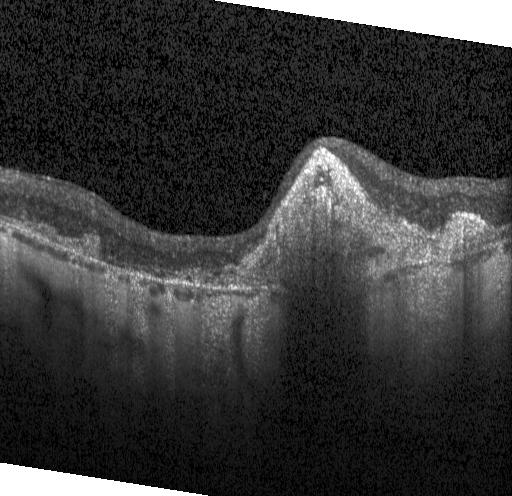

Impression: a choroidal neovascular membrane.